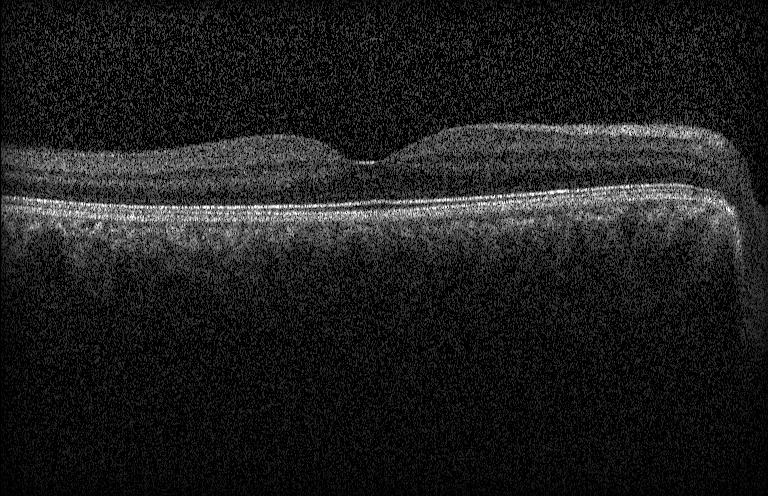

Finding: neither choroidal neovascularization, diabetic macular edema, nor drusen.